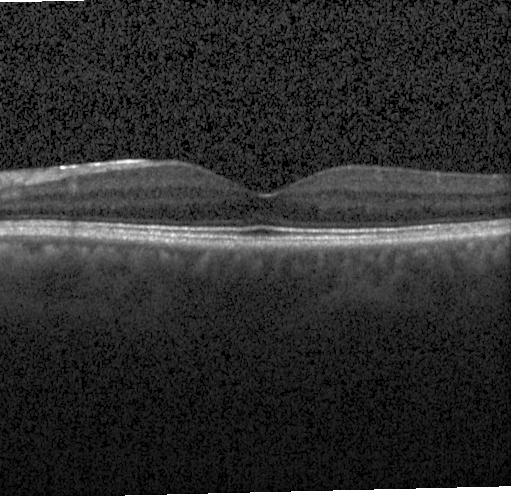
Spectral-domain OCT, fovea-centered, OCT B-scan
OCT finding: neither choroidal neovascularization, diabetic macular edema, nor drusen.